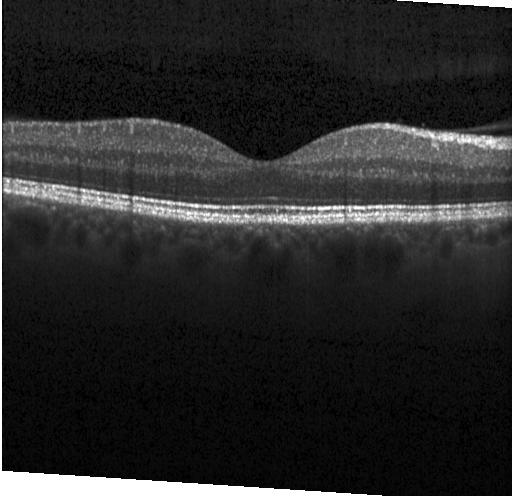 No choroidal neovascularization, no diabetic macular edema, and no drusen.